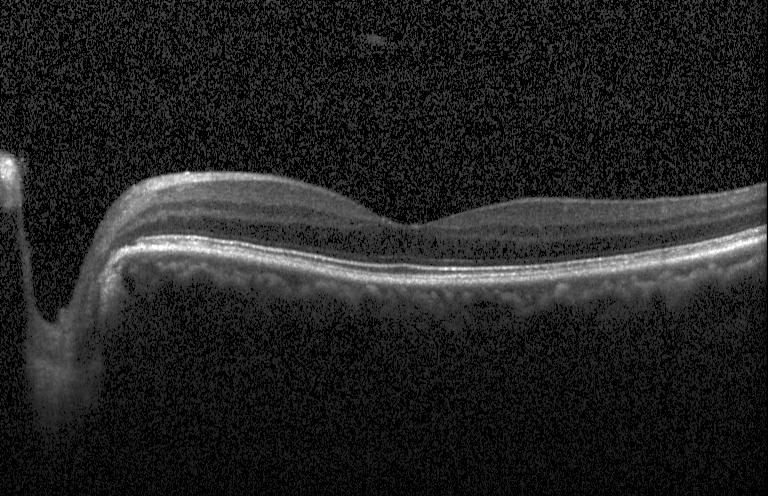 Optical coherence tomography scan. Finding: neither choroidal neovascularization, diabetic macular edema, nor drusen.